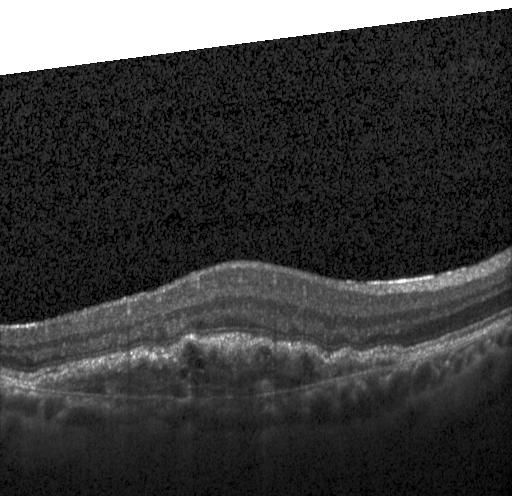 Heidelberg Spectralis; retinal OCT B-scan.
Diagnosis: choroidal neovascularization.